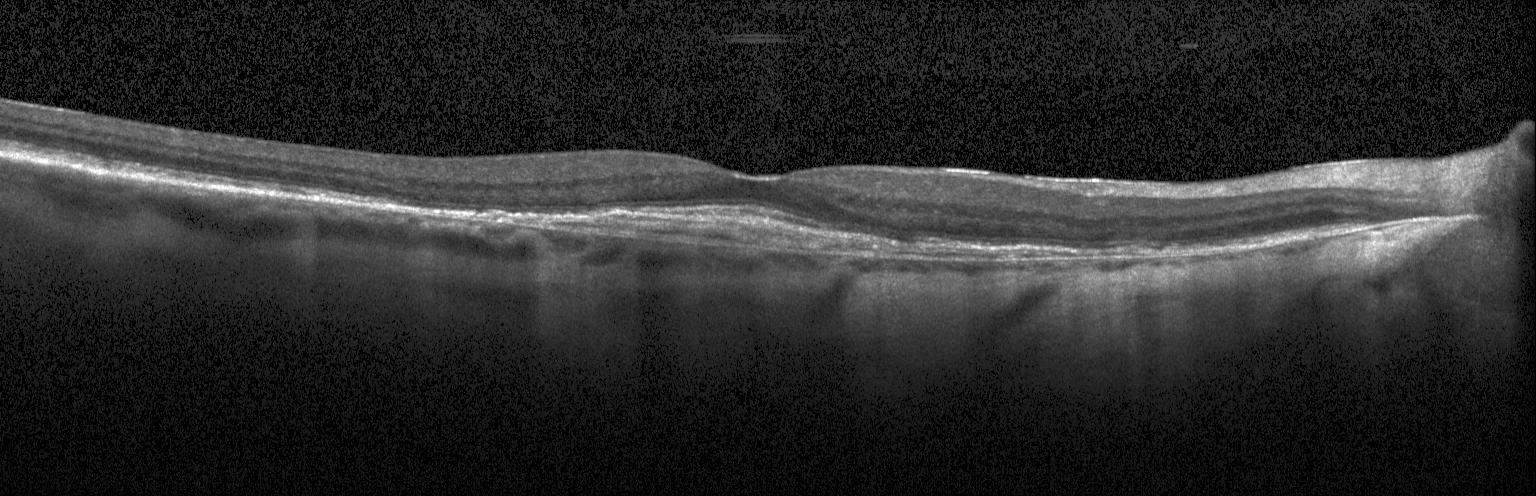 Diagnosis: a choroidal neovascular membrane.